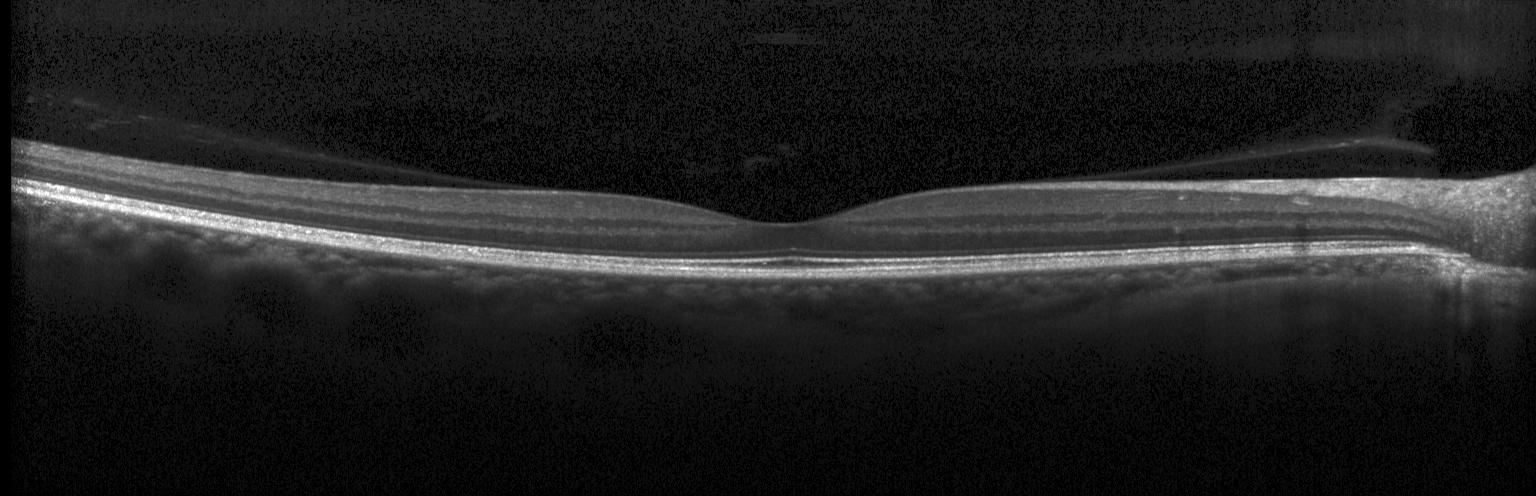
SD-OCT. Retinal OCT cross-section. Heidelberg Spectralis OCT system.
No choroidal neovascularization, no diabetic macular edema, and no drusen.